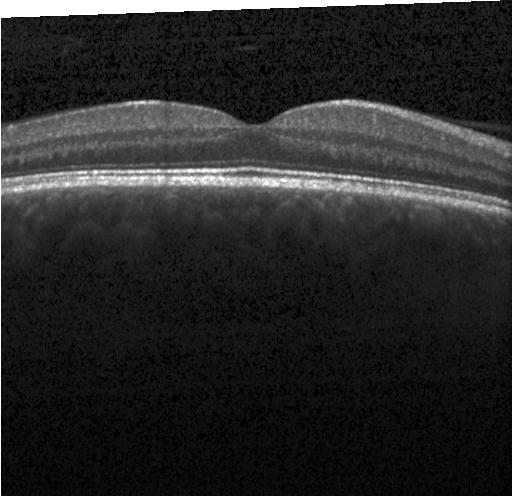
Macular OCT demonstrating no choroidal neovascularization, no diabetic macular edema, and no drusen.